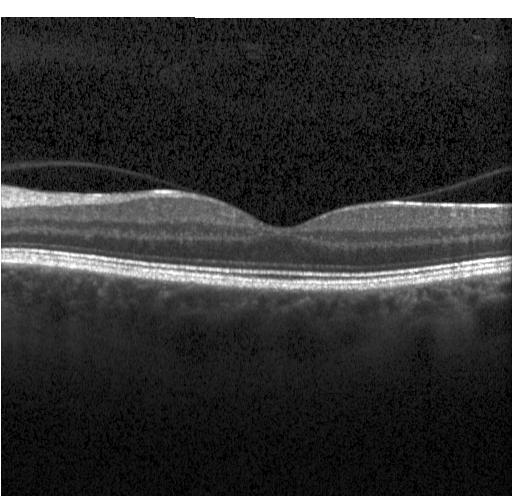

Acquired on a Heidelberg Spectralis, spectral-domain OCT, macular scan, OCT B-scan. Assessment: no choroidal neovascularization, no diabetic macular edema, and no drusen.